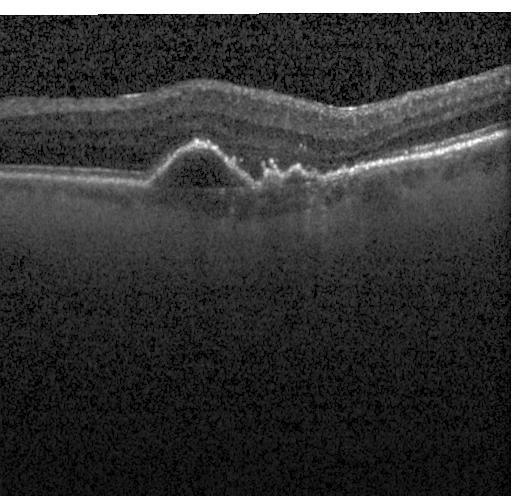

OCT B-scan, SD-OCT, acquired on a Heidelberg Spectralis.
Macular OCT: choroidal neovascularization (CNV).